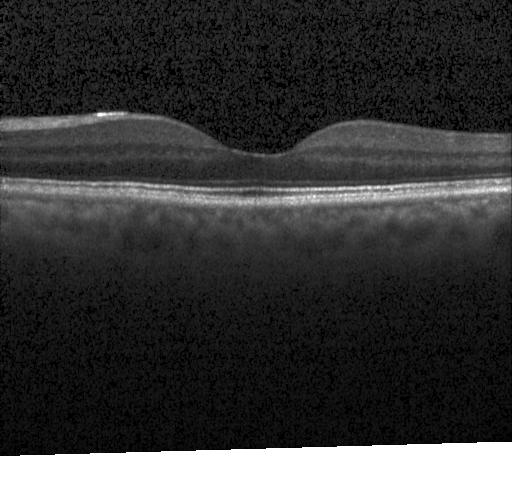 Impression: no choroidal neovascularization, no diabetic macular edema, and no drusen.